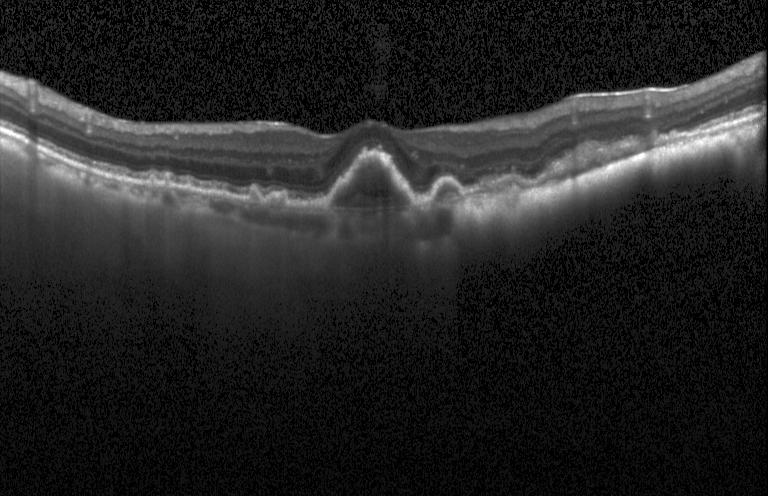 Diagnosis: choroidal neovascularization.